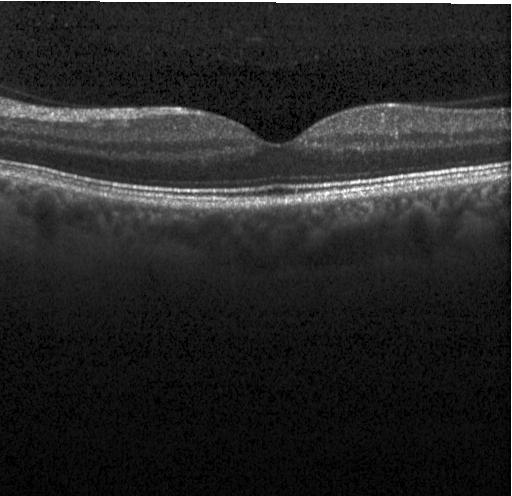

Spectral-domain optical coherence tomography; optical coherence tomography B-scan
The scan shows no choroidal neovascularization, diabetic macular edema, or drusen.